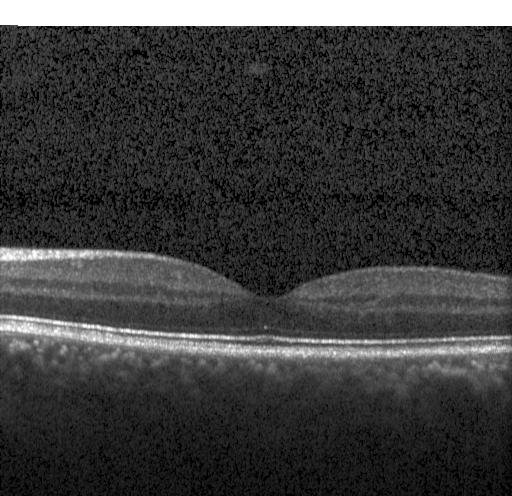

Centered on the fovea; spectral-domain optical coherence tomography; retinal OCT cross-section.
This B-scan demonstrates no choroidal neovascularization, no diabetic macular edema, and no drusen.